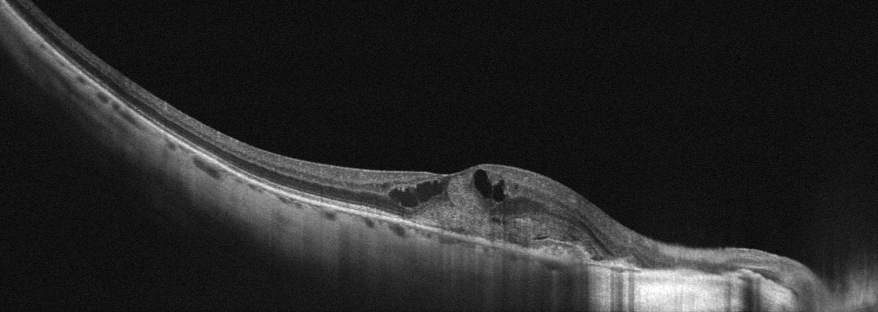

Macular scan. Retinal OCT cross-section. Finding: age-related macular degeneration (AMD).